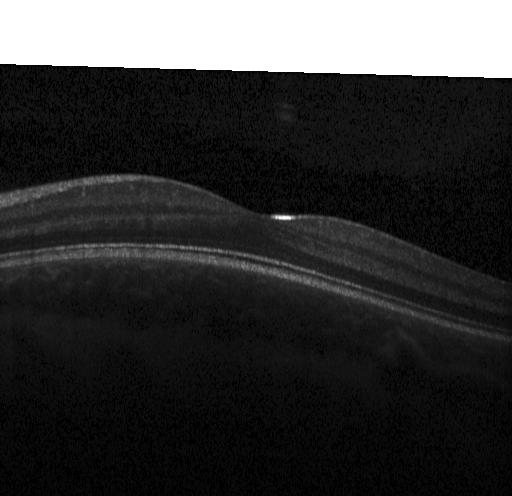

OCT B-scan showing no choroidal neovascularization, no diabetic macular edema, and no drusen.